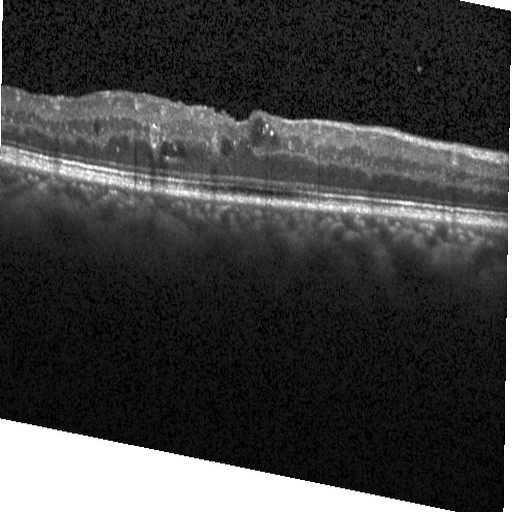

Diagnosis: diabetic macular edema.